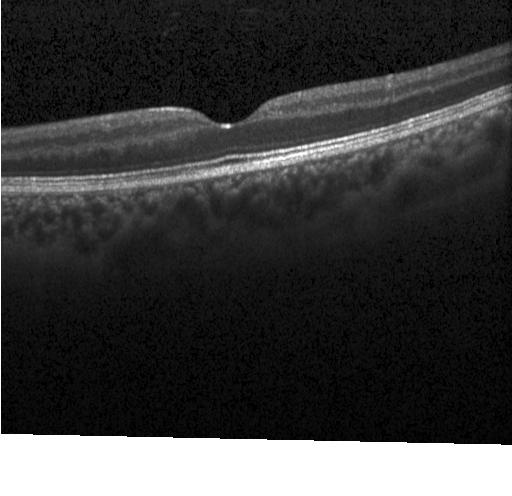 Heidelberg Spectralis, retinal OCT cross-section — The scan shows neither CNV, DME, nor drusen.